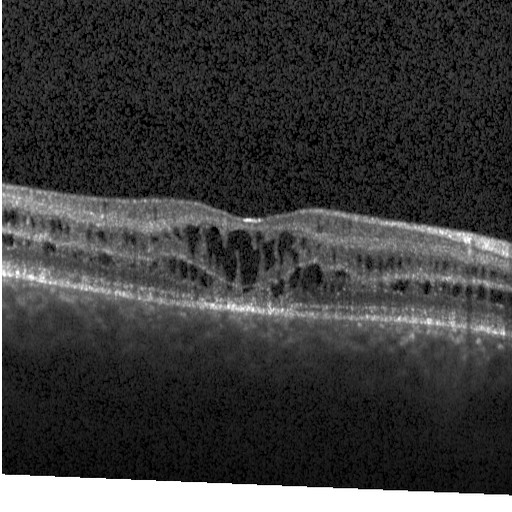
Retinal OCT cross-section.
Diabetic macular edema.